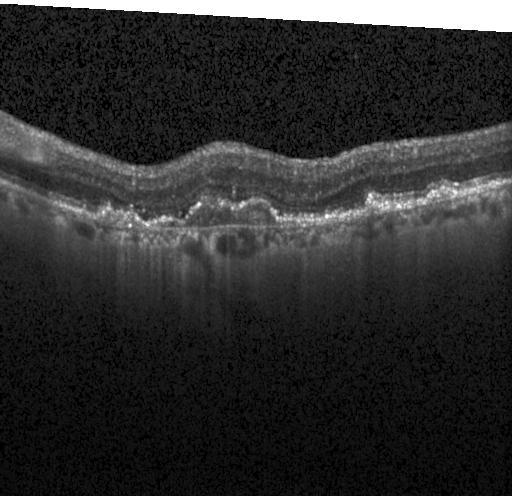
OCT B-scan · acquired on a Heidelberg Spectralis · spectral-domain optical coherence tomography · through the macula — Diagnosis: a choroidal neovascular membrane.